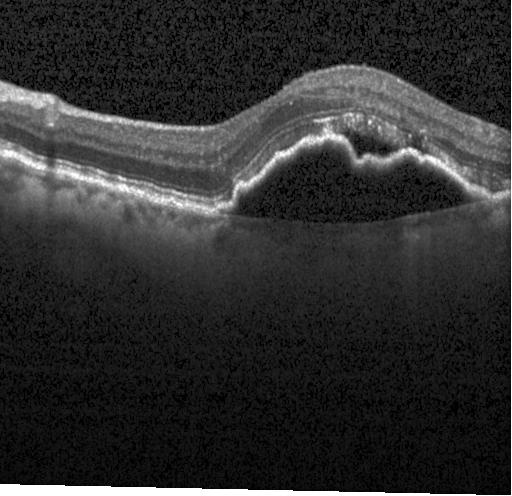
OCT B-scan showing a choroidal neovascular membrane.